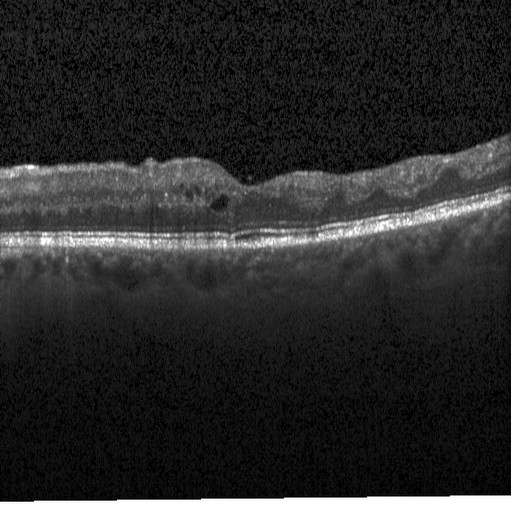
OCT finding: DME.